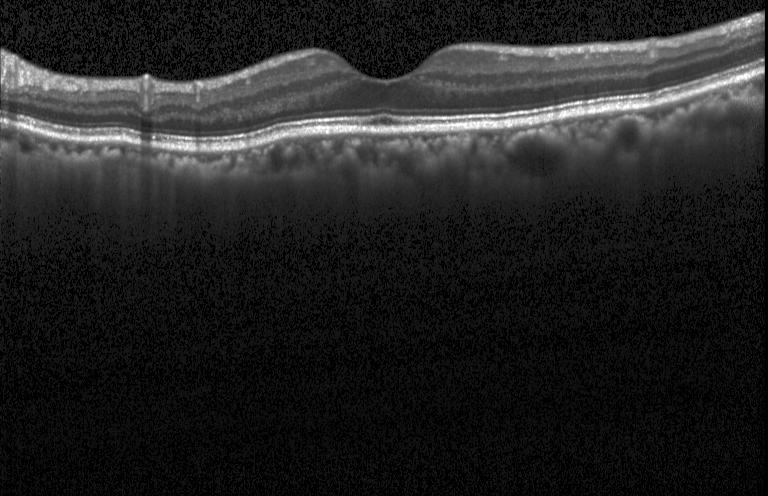 This B-scan demonstrates neither choroidal neovascularization, diabetic macular edema, nor drusen.